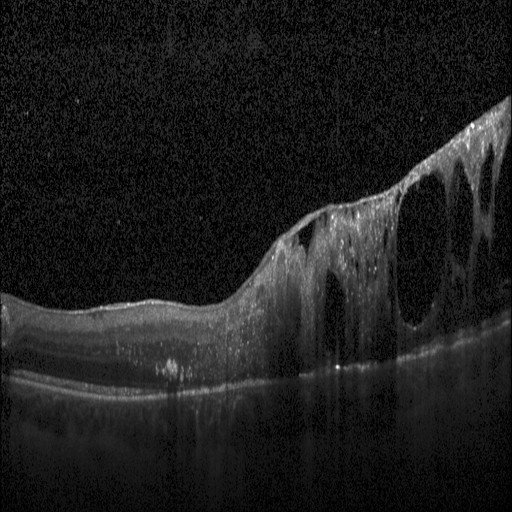 The scan shows diabetic macular edema.